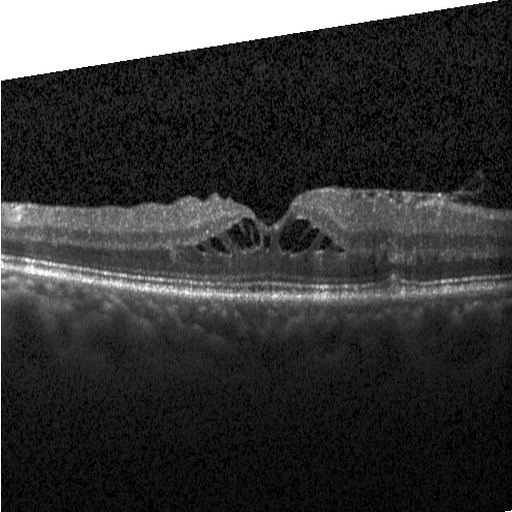

Spectral-domain OCT. Optical coherence tomography scan. Instrument: Heidelberg Spectralis. Centered on the fovea
Diabetic macular edema (DME).